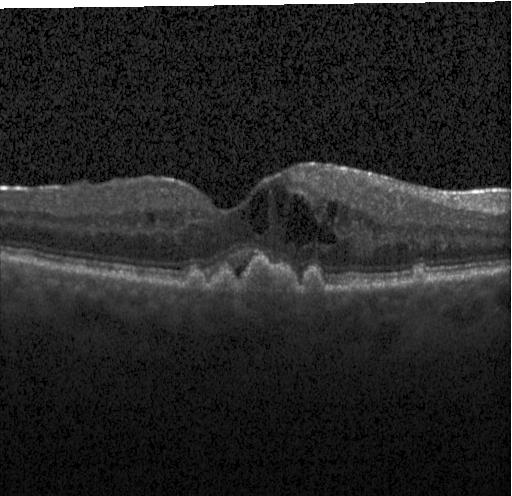

OCT line scan. Assessment: choroidal neovascularization.